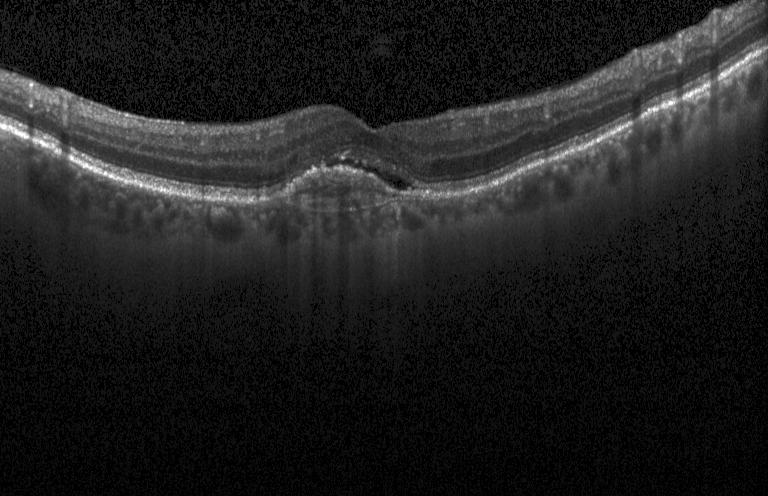
Dx: a choroidal neovascular membrane.